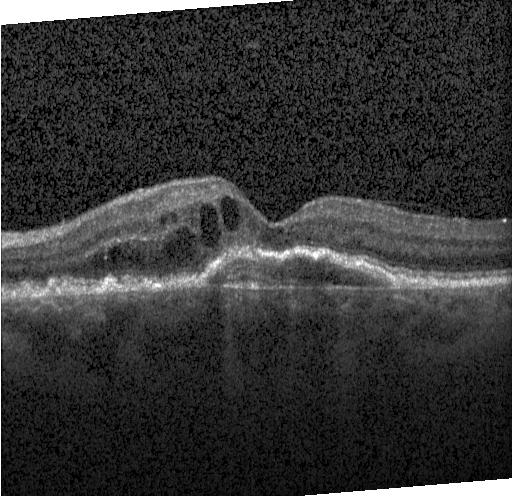

Heidelberg Spectralis, spectral-domain optical coherence tomography, OCT line scan. A choroidal neovascular membrane.